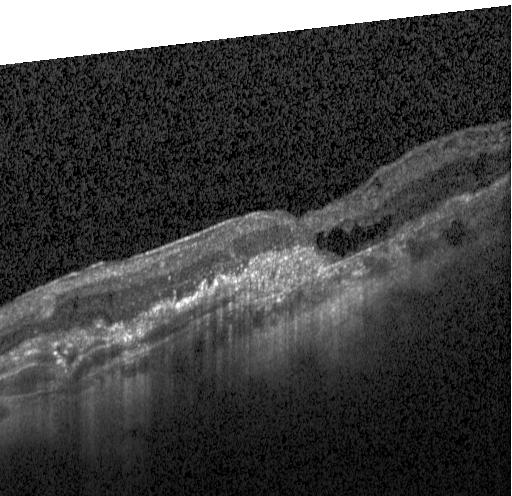

The scan shows a choroidal neovascular membrane.